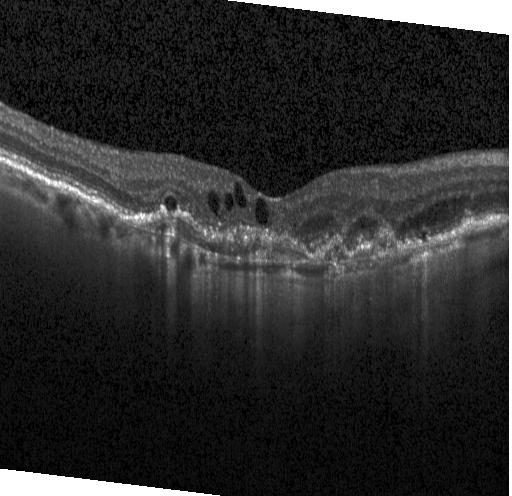

Finding: CNV.